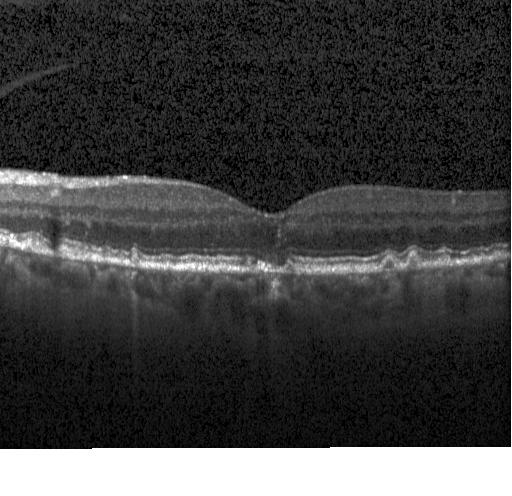 OCT B-scan showing multiple drusen.